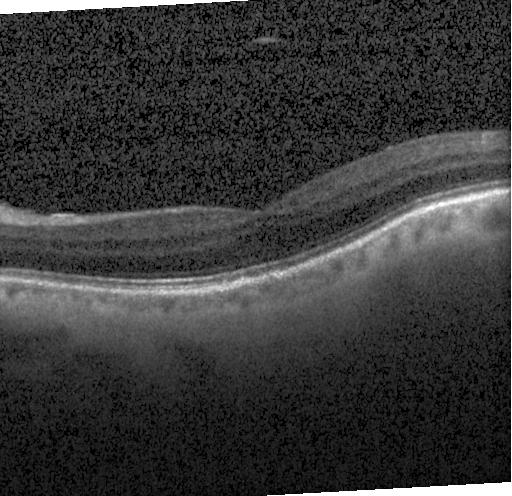 Impression: neither choroidal neovascularization, diabetic macular edema, nor drusen.